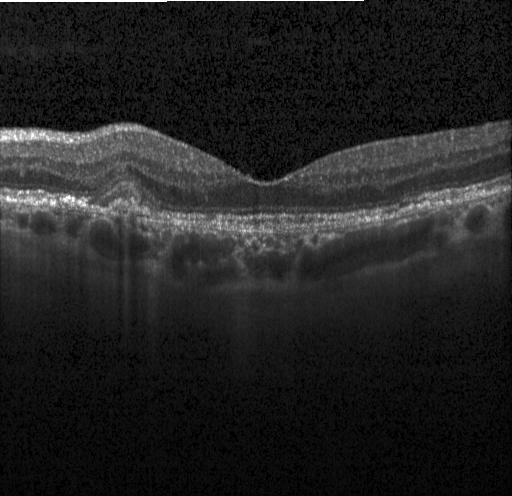
Macular scan, OCT line scan
OCT finding: sub-RPE drusenoid deposits.